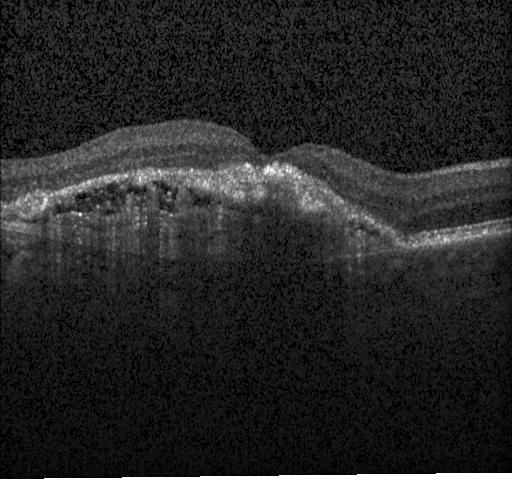 Acquired on a Heidelberg Spectralis, through the macula, retinal OCT cross-section
Assessment: a choroidal neovascular membrane.